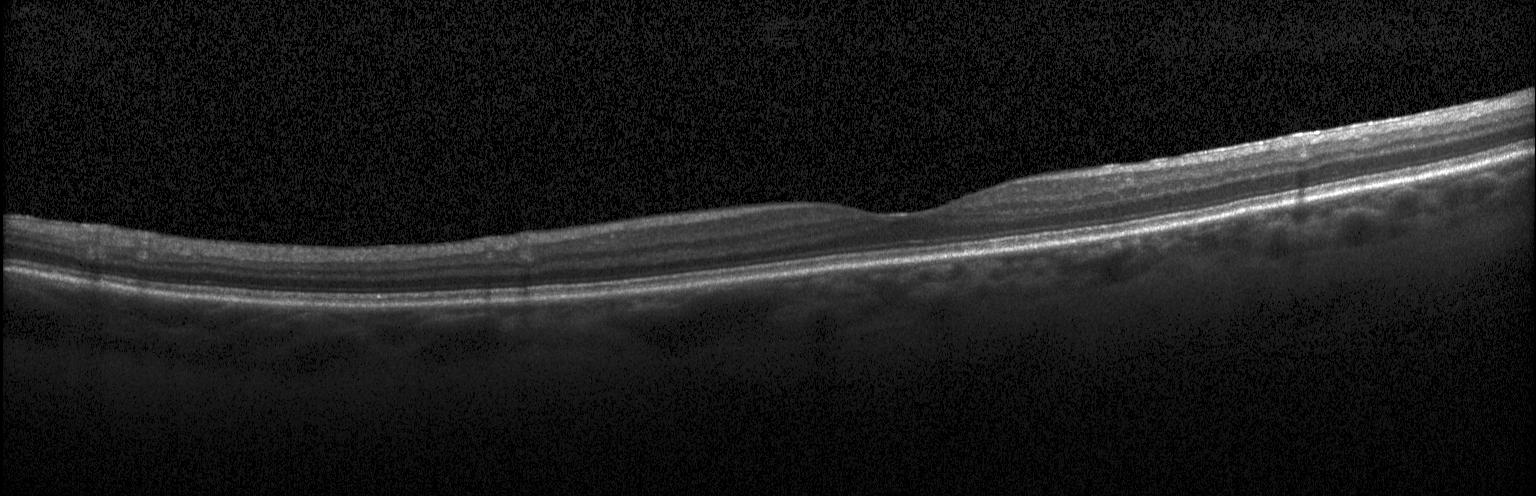 Heidelberg Spectralis. OCT B-scan
Finding: no choroidal neovascularization, diabetic macular edema, or drusen.